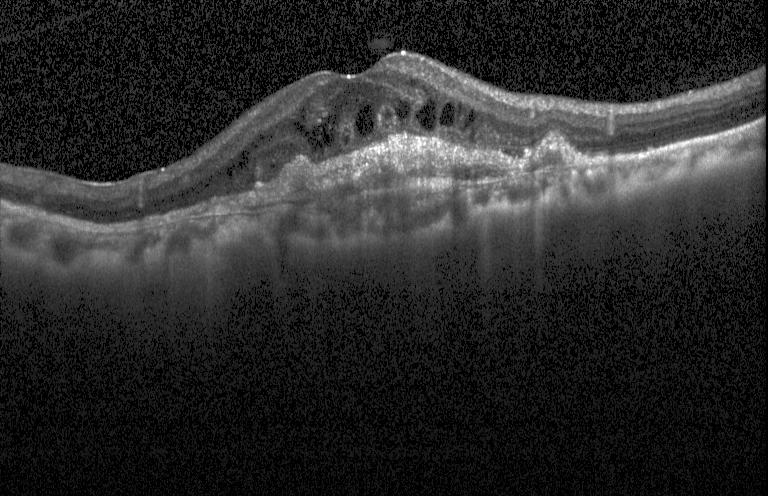

This B-scan demonstrates CNV.